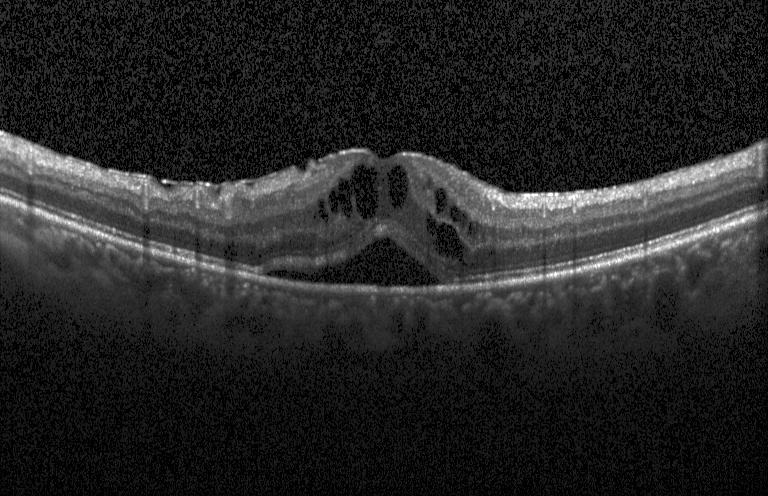
Optical coherence tomography B-scan · acquired on a Heidelberg Spectralis · fovea-centered.
Finding: DME.